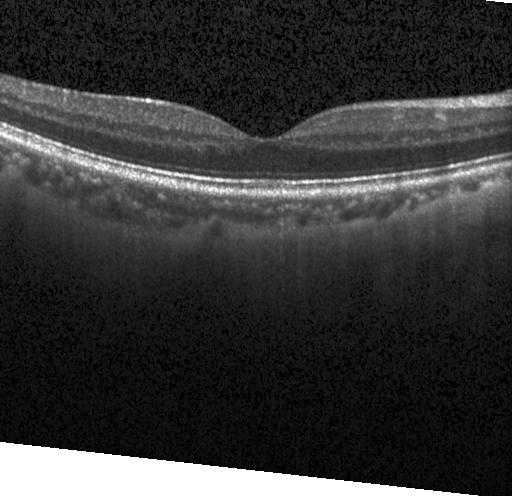

Macular OCT: no choroidal neovascularization, diabetic macular edema, or drusen.